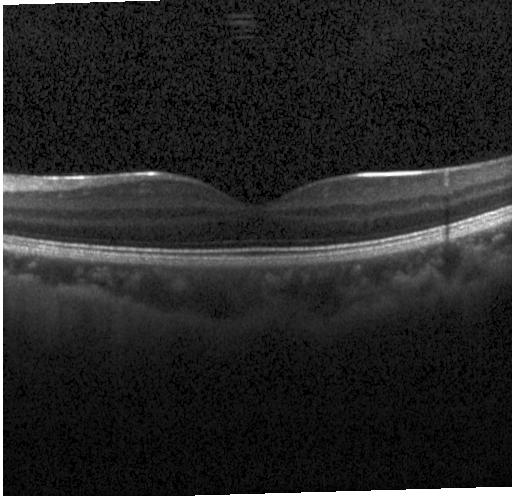

Through the macula. Optical coherence tomography scan — Impression: no CNV, DME, or drusen.